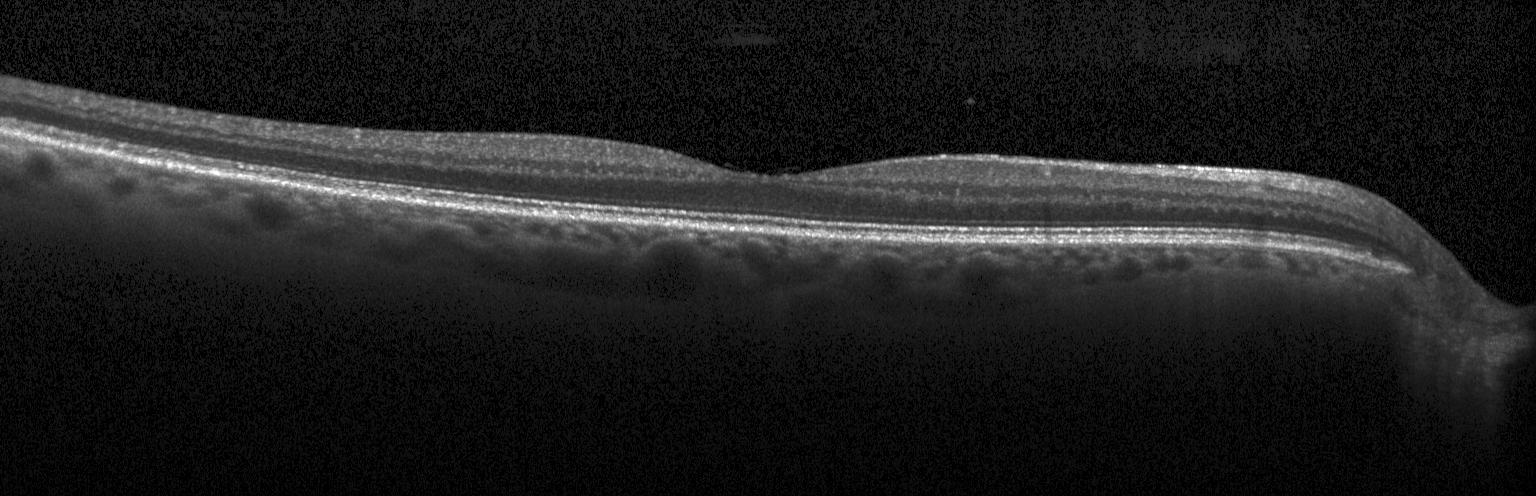

Retinal OCT cross-section showing no evidence of choroidal neovascularization, diabetic macular edema, or drusen.